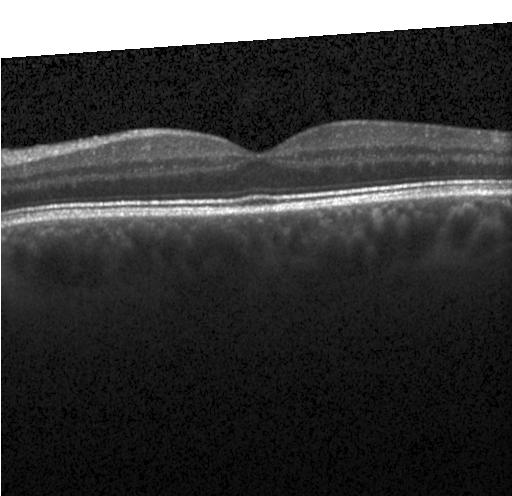

Centered on the fovea; SD-OCT; optical coherence tomography scan — Macular OCT: no CNV, no DME, and no drusen.